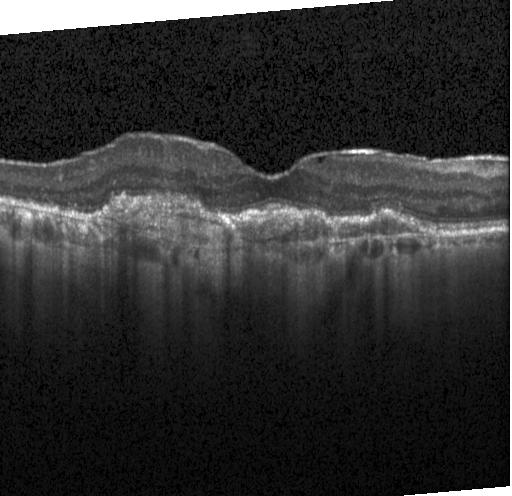
Centered on the fovea. Retinal OCT cross-section. Acquired on a Heidelberg Spectralis — A choroidal neovascular membrane.